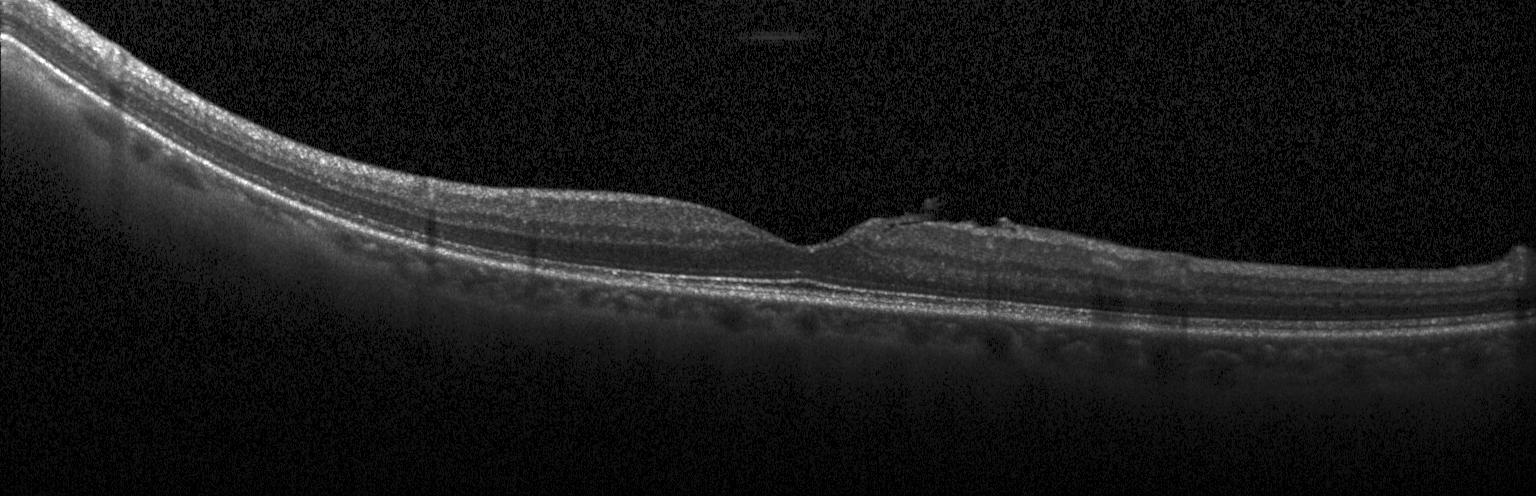

Assessment: no choroidal neovascularization, diabetic macular edema, or drusen.